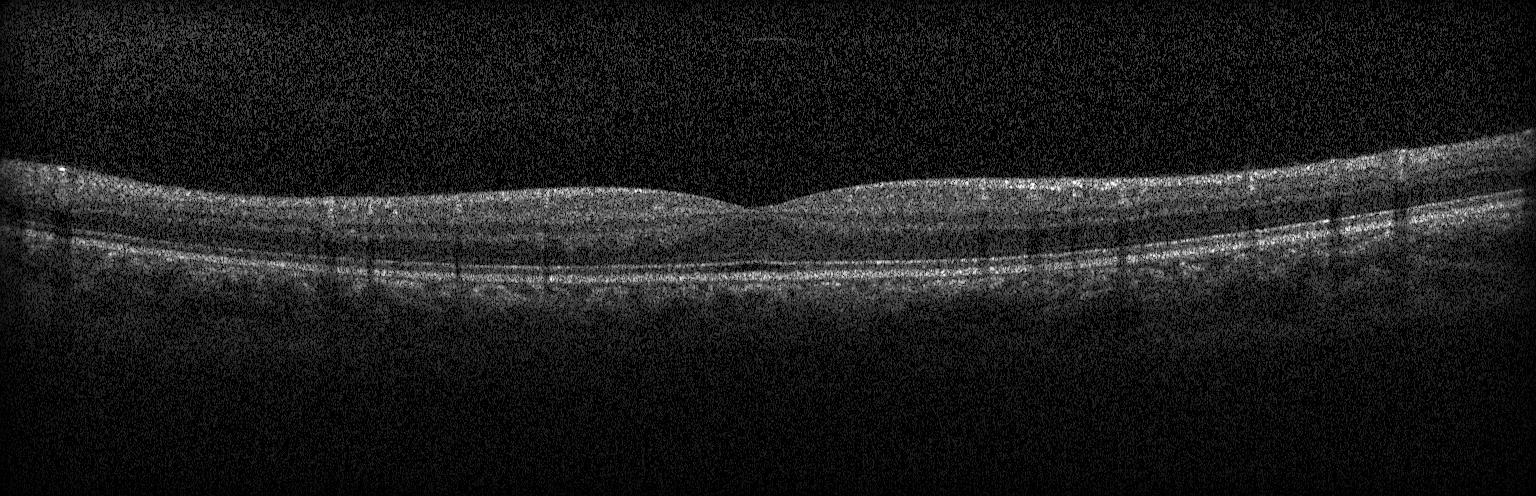
Retinal OCT cross-section
This B-scan demonstrates no CNV, DME, or drusen.